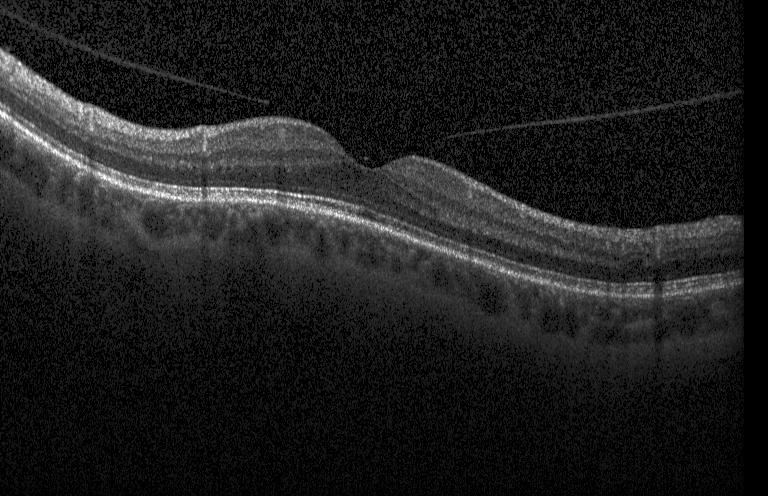

Optical coherence tomography scan; through the macula; Heidelberg Spectralis.
Diagnosis: no evidence of choroidal neovascularization, diabetic macular edema, or drusen.